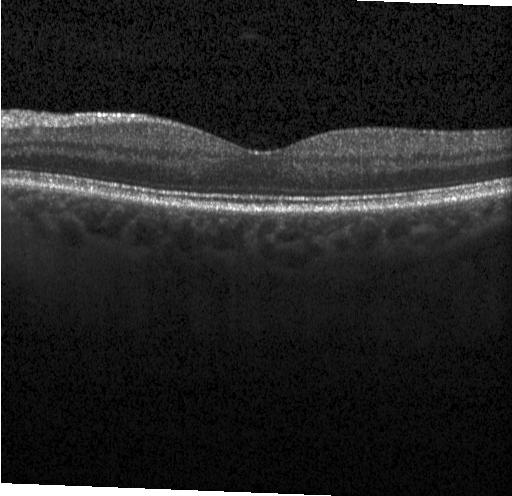 OCT finding: no choroidal neovascularization, no diabetic macular edema, and no drusen.